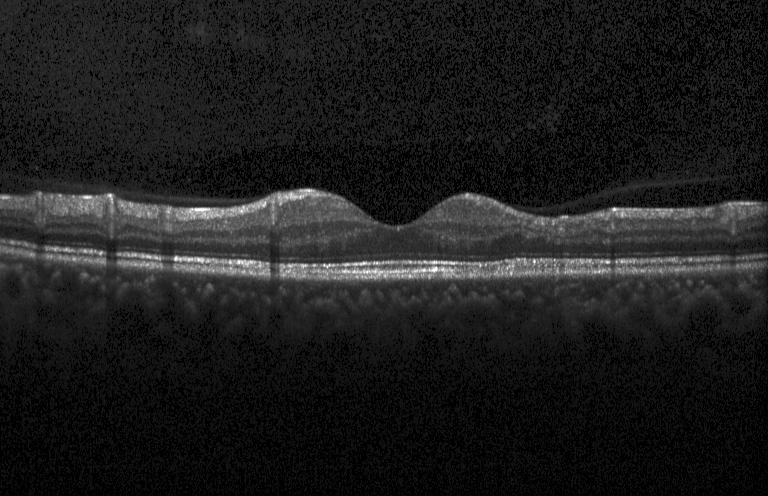
OCT B-scan showing no choroidal neovascularization, diabetic macular edema, or drusen.